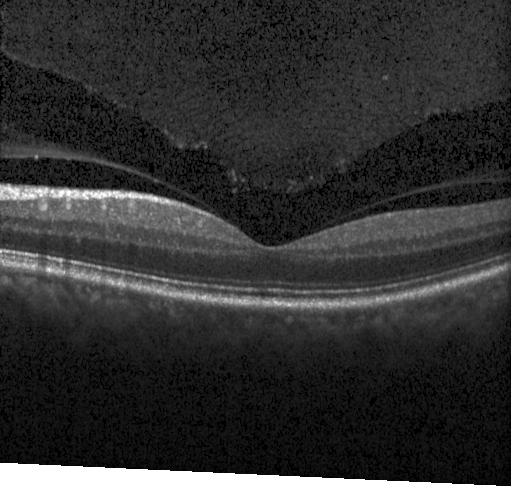

Dx: no evidence of choroidal neovascularization, diabetic macular edema, or drusen.